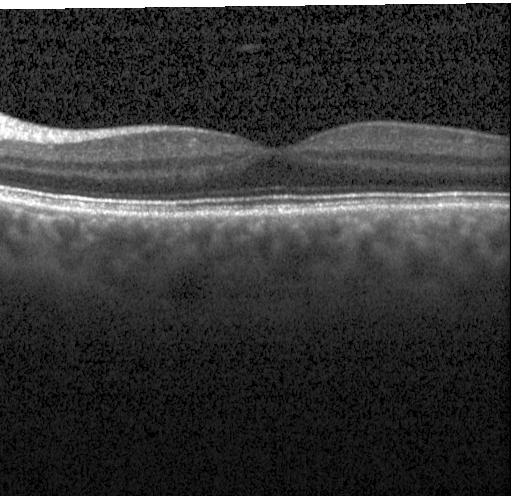 Retinal OCT cross-section — Impression: neither choroidal neovascularization, diabetic macular edema, nor drusen.